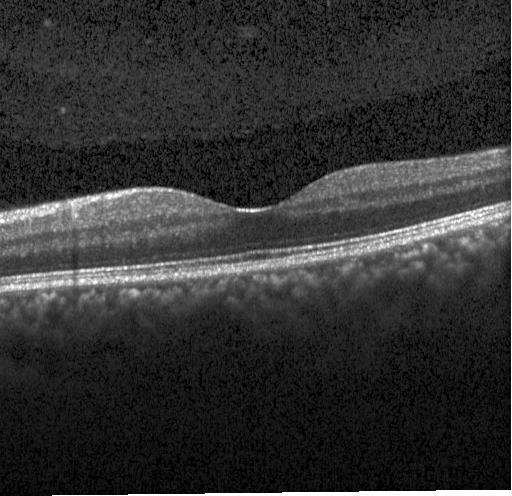

Retinal OCT B-scan — Assessment: no CNV, no DME, and no drusen.